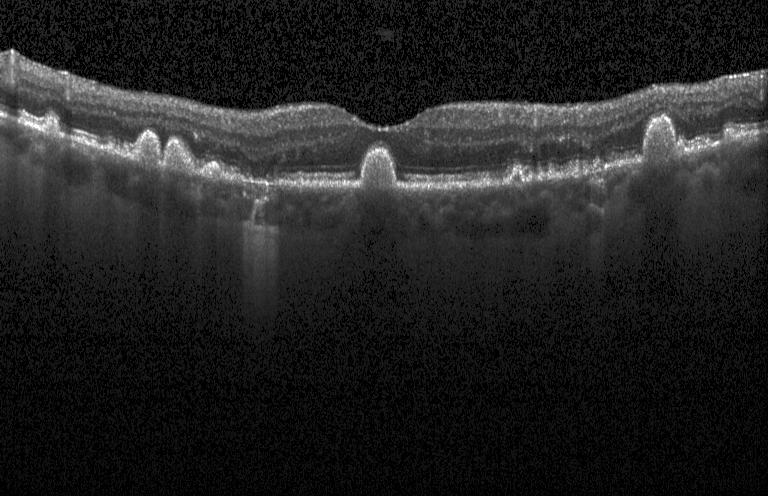

OCT B-scan.
This B-scan demonstrates sub-RPE drusenoid deposits.